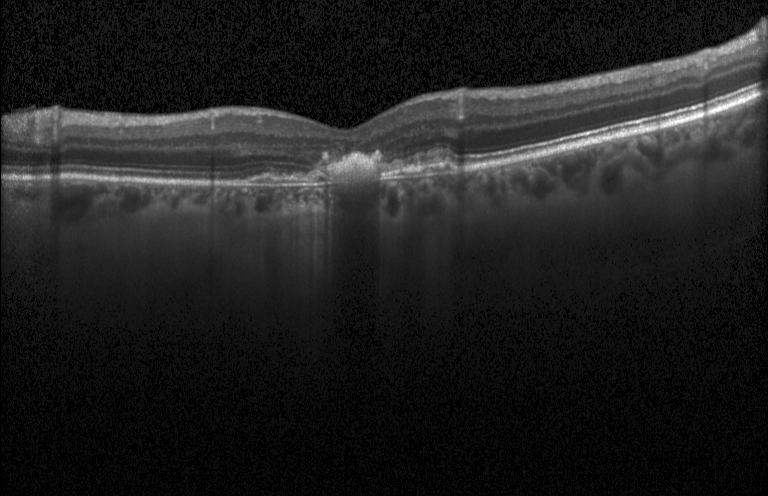

The scan shows a choroidal neovascular membrane.